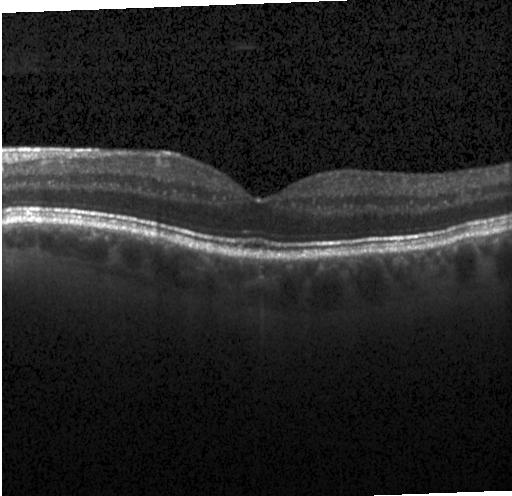 Dx: no choroidal neovascularization, no diabetic macular edema, and no drusen.